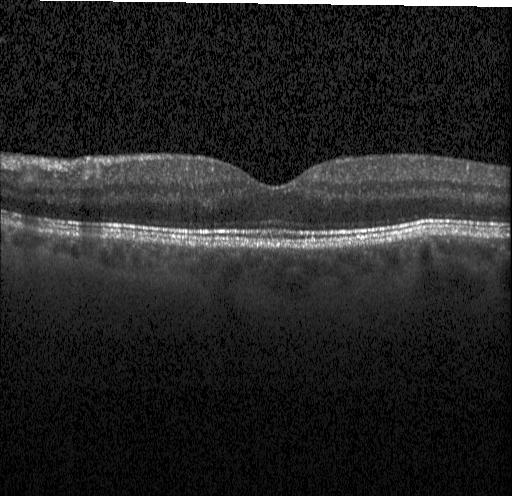

Optical coherence tomography scan. Through the macula — Macular OCT: neither CNV, DME, nor drusen.